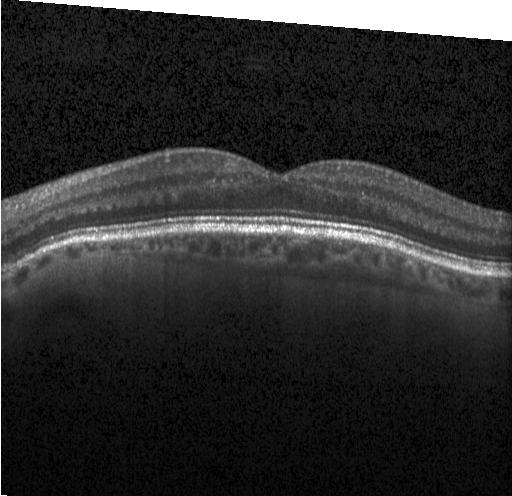

Fovea-centered. Retinal OCT cross-section
Dx: no evidence of CNV, DME, or drusen.